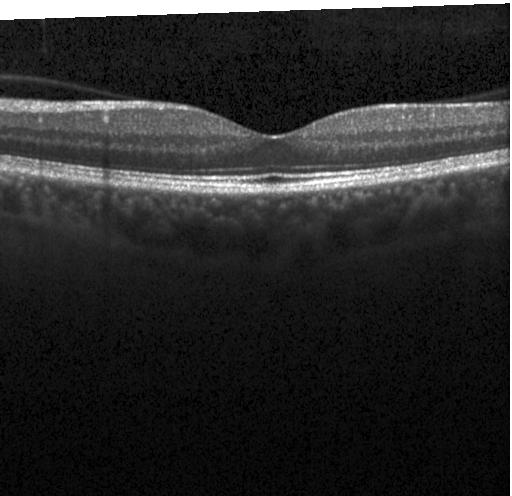
Heidelberg Spectralis · OCT B-scan. Macular OCT: no choroidal neovascularization, no diabetic macular edema, and no drusen.